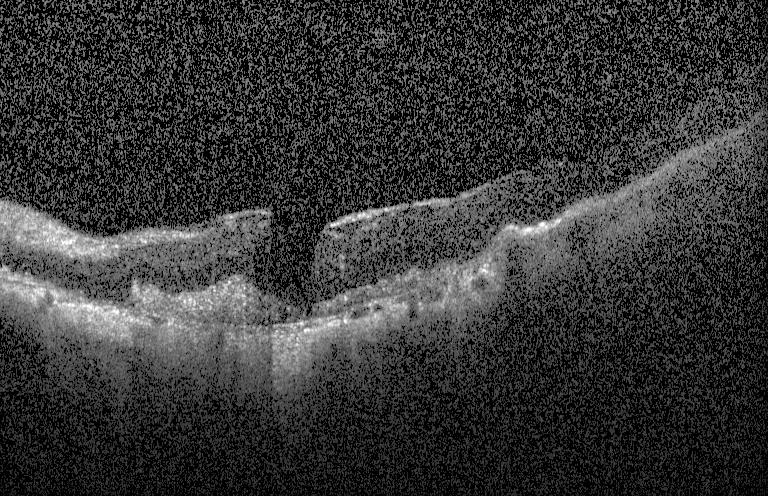 Finding: a choroidal neovascular membrane.